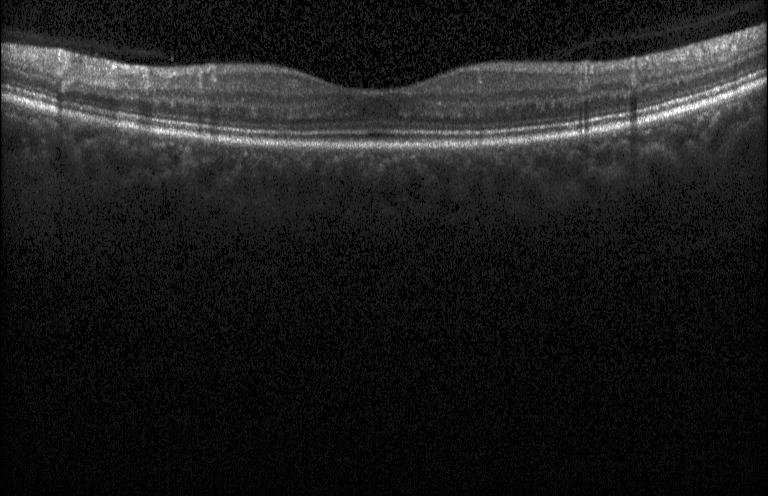 Finding: no evidence of choroidal neovascularization, diabetic macular edema, or drusen.